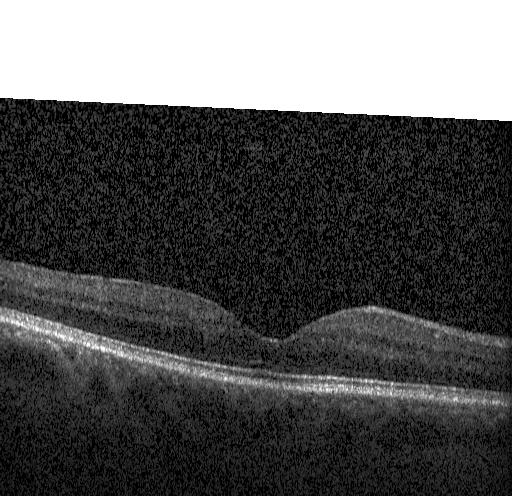 The scan shows no CNV, DME, or drusen.